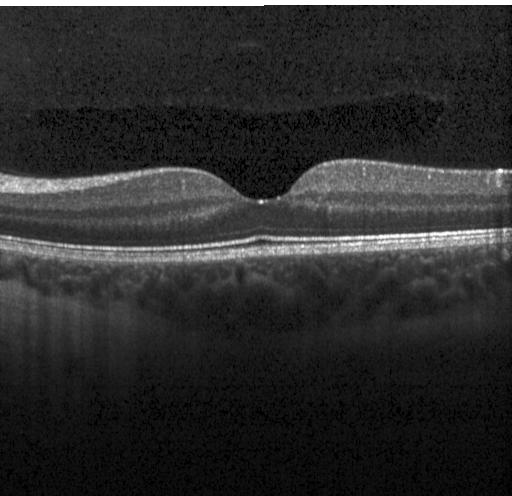
OCT B-scan · horizontal scan through the fovea · Heidelberg Spectralis OCT system
Assessment: no evidence of CNV, DME, or drusen.